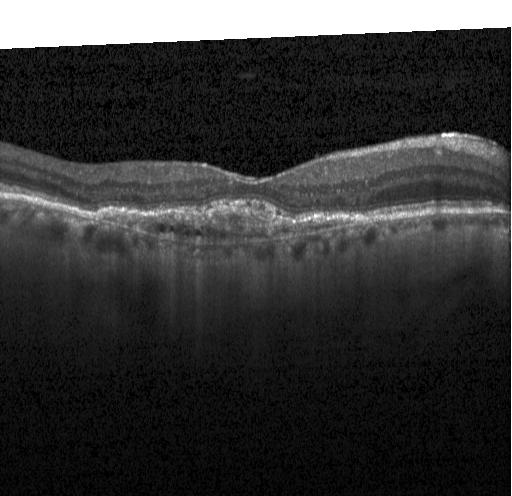
Diagnosis: a choroidal neovascular membrane.